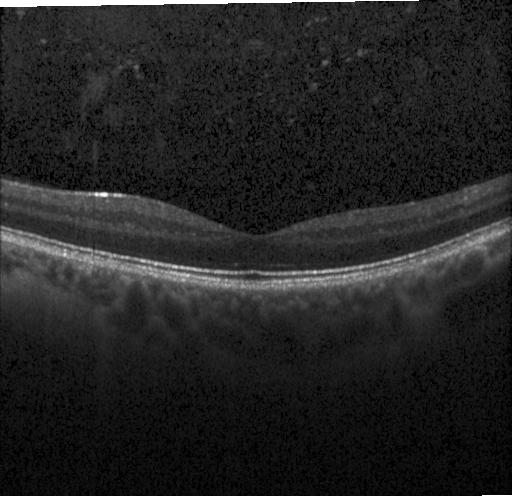
Diagnosis: no evidence of choroidal neovascularization, diabetic macular edema, or drusen.